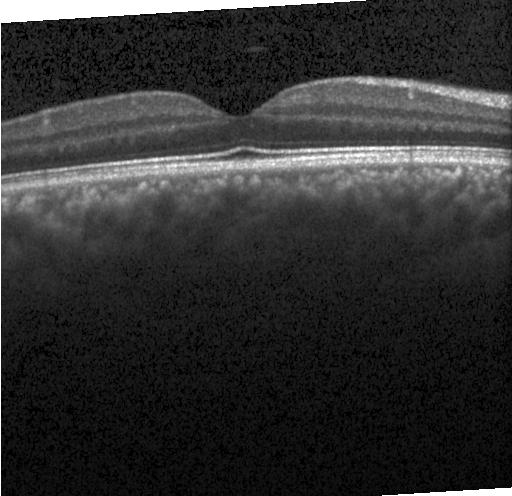
OCT line scan; instrument: Heidelberg Spectralis; spectral-domain OCT — Finding: no CNV, no DME, and no drusen.